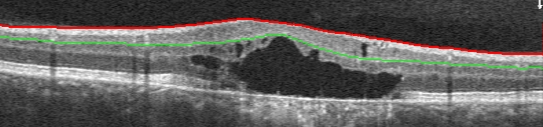

Acquired on an Optovue Avanti RTVue XR; OCT line scan; through the macula — Impression: AMD.